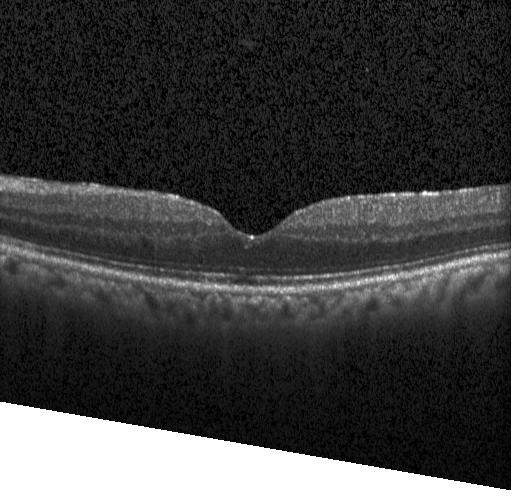 Horizontal scan through the fovea · Heidelberg Spectralis · SD-OCT · optical coherence tomography B-scan. Finding: no choroidal neovascularization, diabetic macular edema, or drusen.